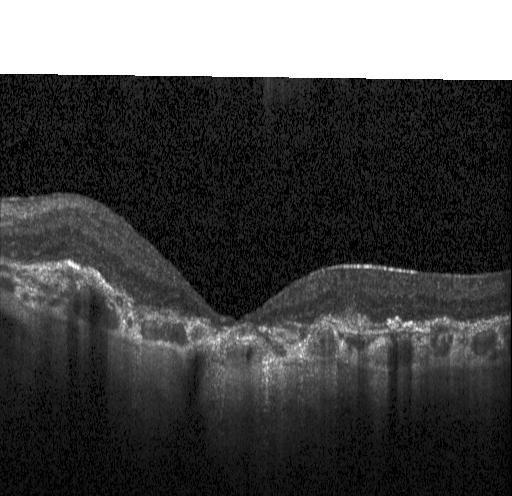
Retinal OCT cross-section, spectral-domain OCT, centered on the fovea, instrument: Heidelberg Spectralis — Dx: CNV.